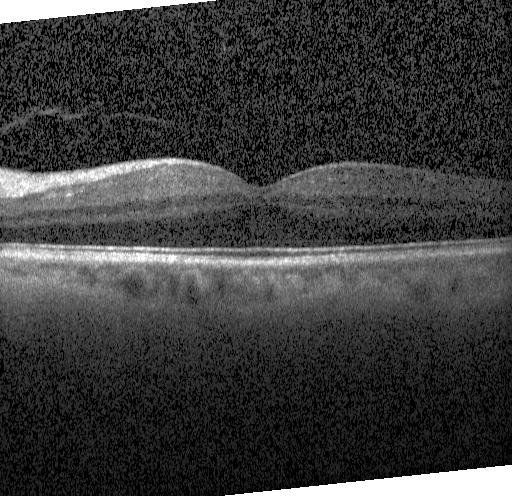
Centered on the fovea. Instrument: Heidelberg Spectralis. SD-OCT. Retinal OCT B-scan. Impression: no evidence of choroidal neovascularization, diabetic macular edema, or drusen.